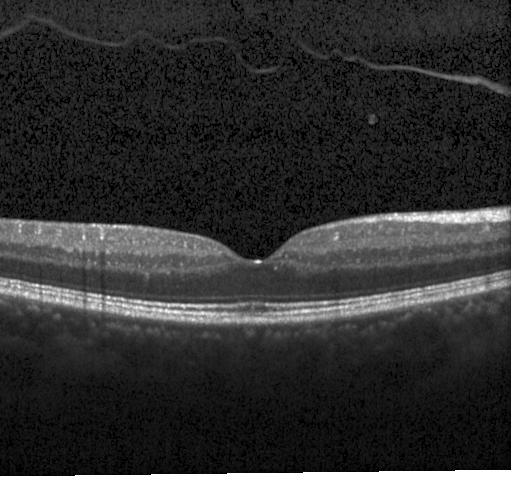
Spectral-domain OCT B-scan: no choroidal neovascularization, no diabetic macular edema, and no drusen.